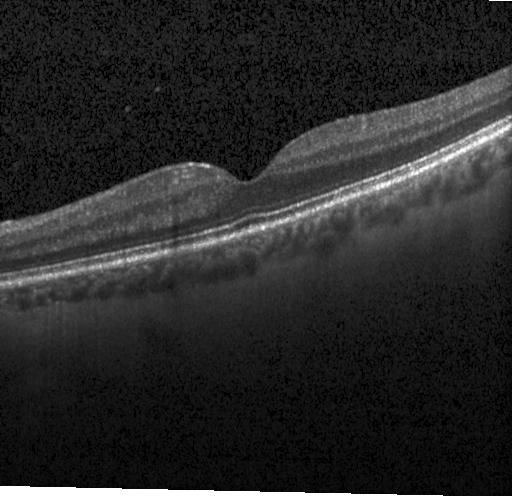

Finding: no evidence of choroidal neovascularization, diabetic macular edema, or drusen.